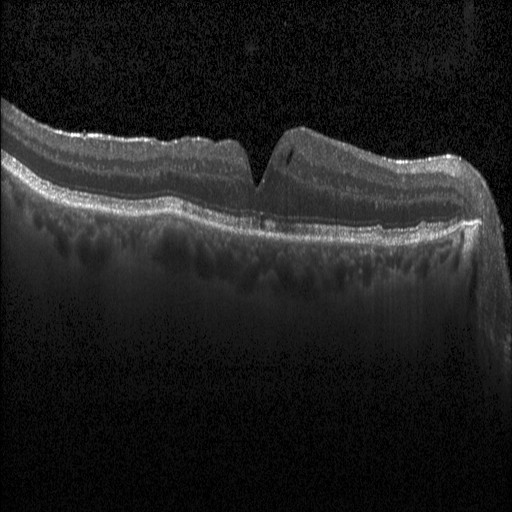

Macular OCT: DME.